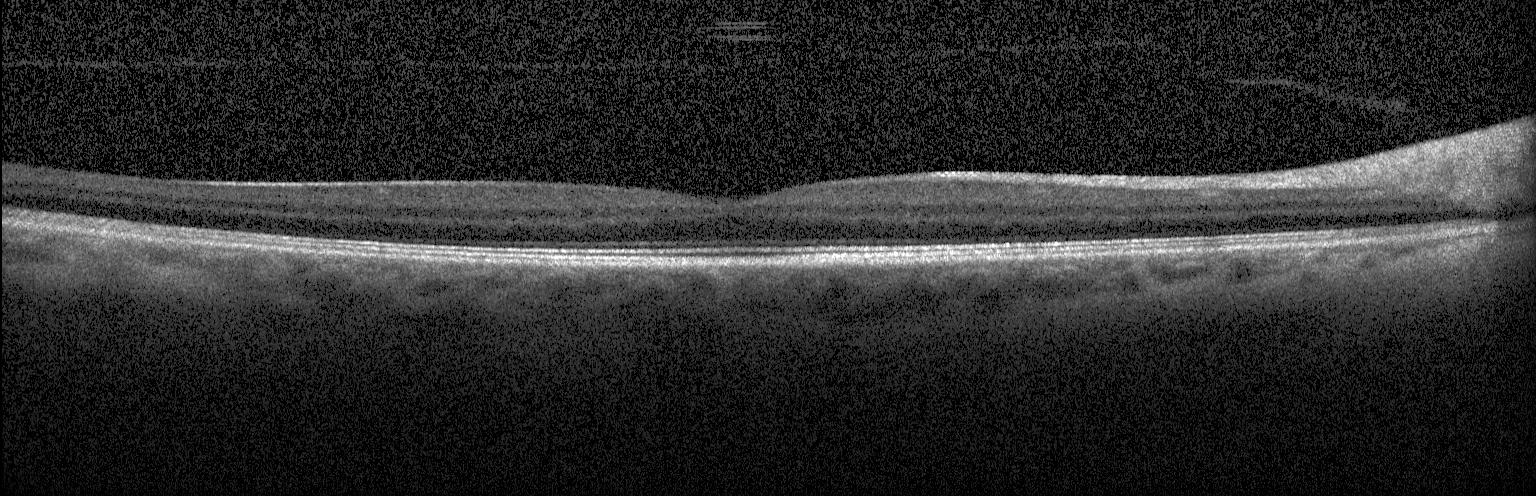 OCT finding: no evidence of choroidal neovascularization, diabetic macular edema, or drusen.